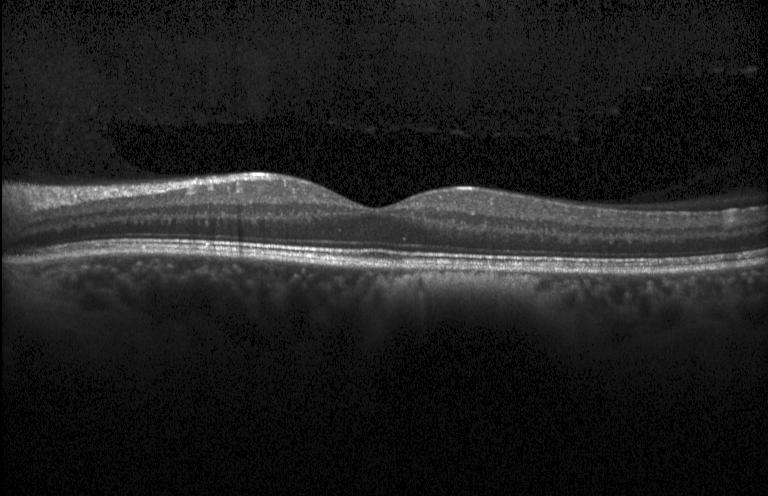

OCT B-scan.
OCT finding: neither choroidal neovascularization, diabetic macular edema, nor drusen.